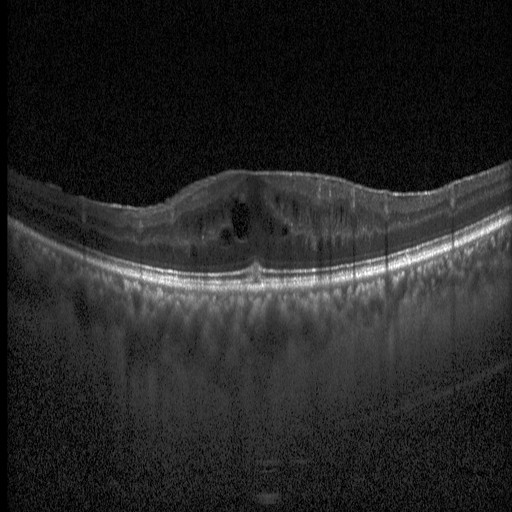

Instrument: Heidelberg Spectralis; retinal OCT B-scan. Diagnosis: diabetic macular edema (DME).